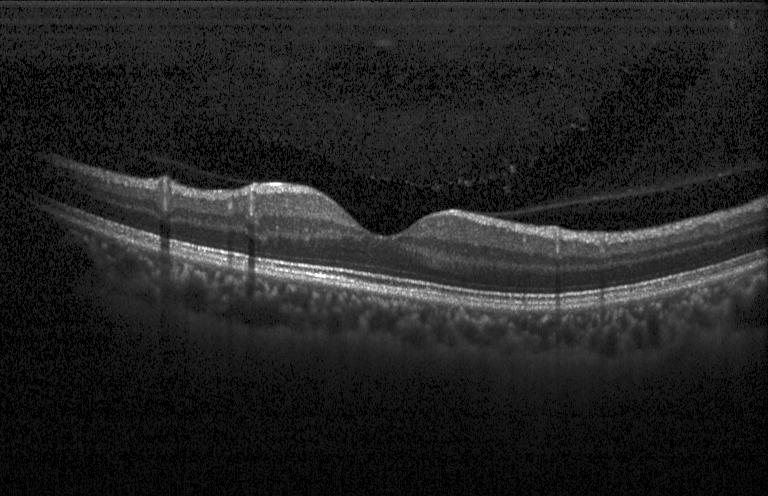

Macular OCT: neither choroidal neovascularization, diabetic macular edema, nor drusen.